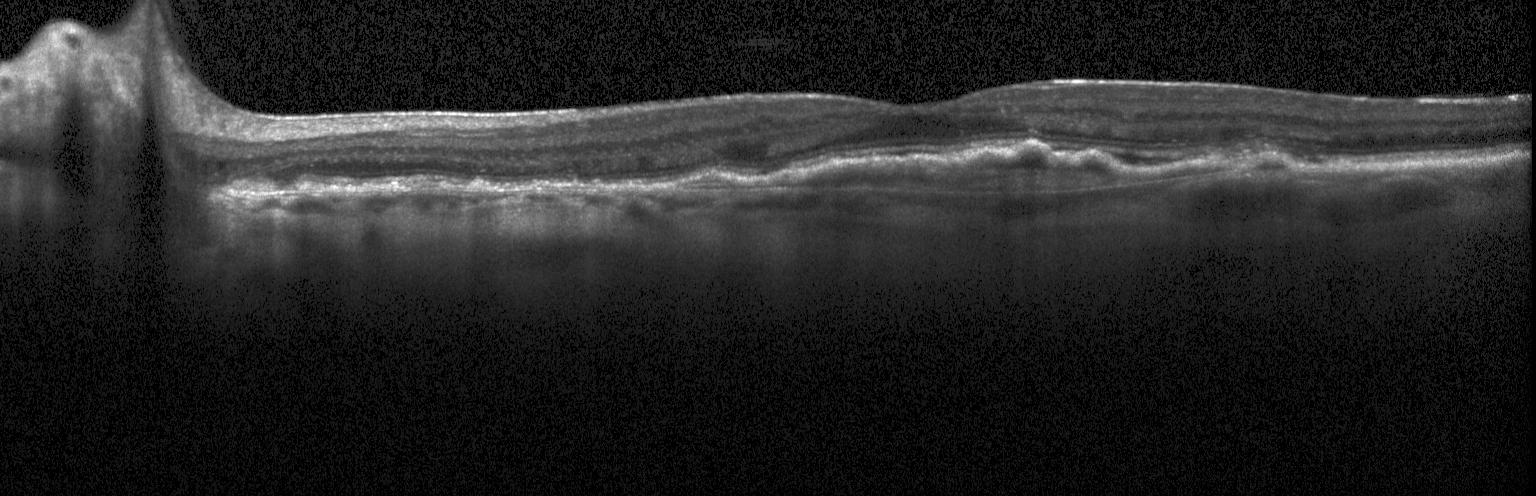
Diagnosis: a choroidal neovascular membrane.